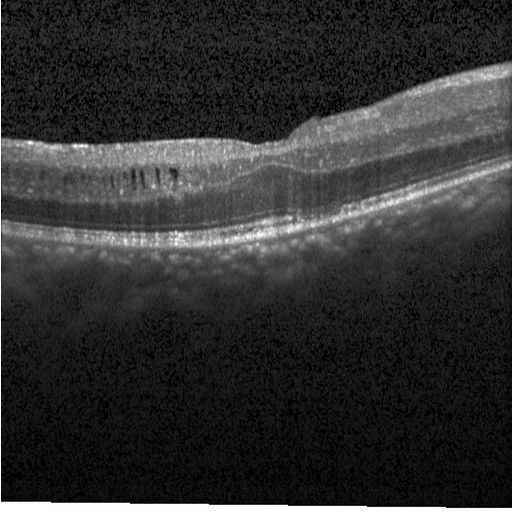 Optical coherence tomography B-scan. Assessment: diabetic macular edema.